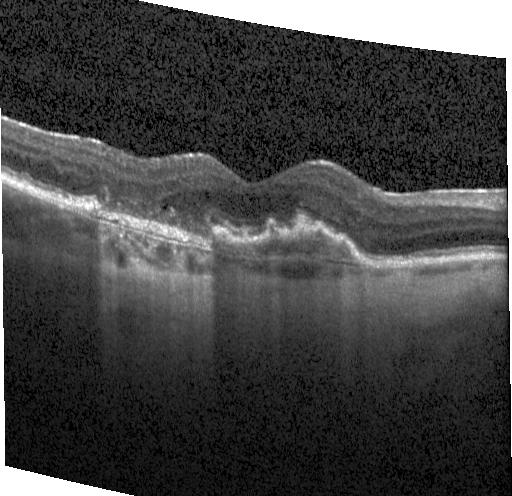 Dx: a choroidal neovascular membrane.